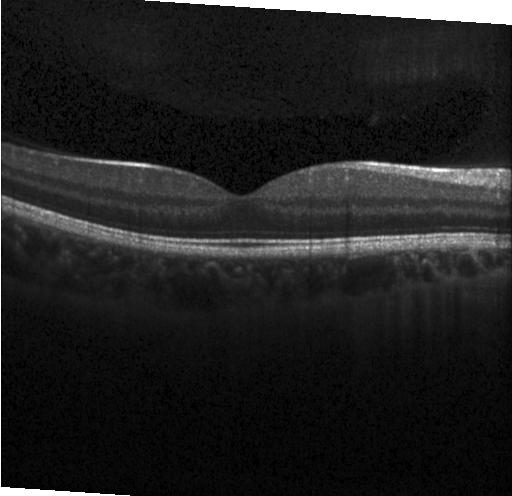 OCT line scan; spectral-domain optical coherence tomography; fovea-centered
Assessment: neither choroidal neovascularization, diabetic macular edema, nor drusen.